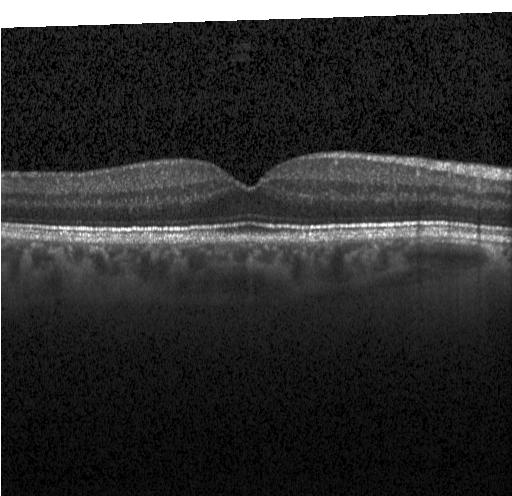
OCT finding: no CNV, DME, or drusen.